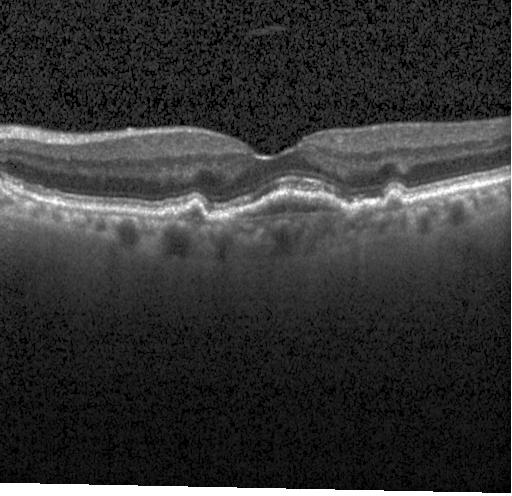 Centered on the fovea · optical coherence tomography scan · acquired on a Heidelberg Spectralis · SD-OCT
Diagnosis: choroidal neovascularization (CNV).